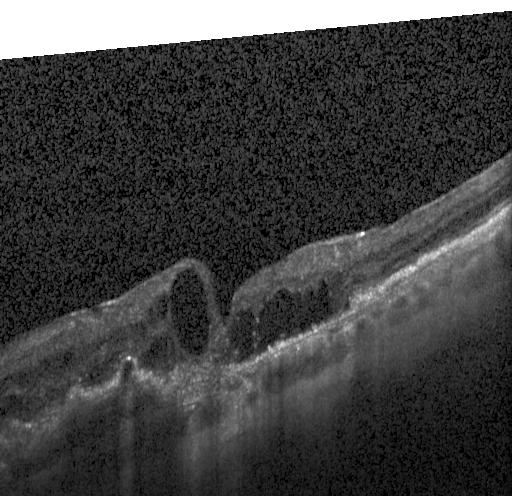 Assessment: CNV.